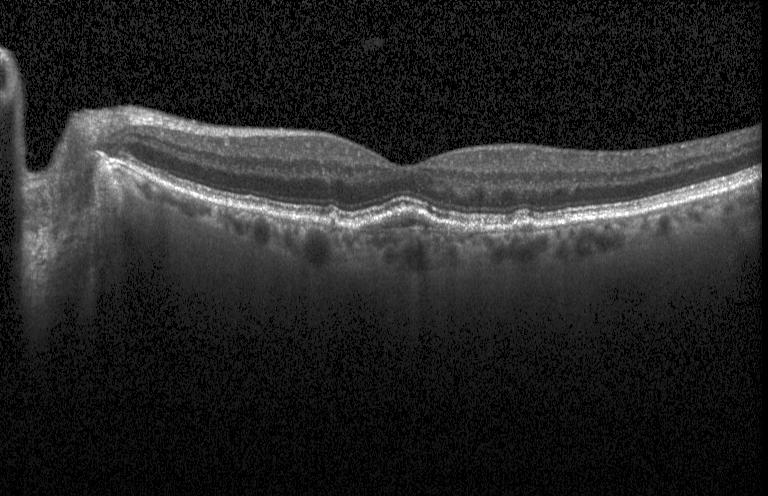 Macular scan; retinal OCT cross-section; SD-OCT; Heidelberg Spectralis
Diagnosis: choroidal neovascularization (CNV).